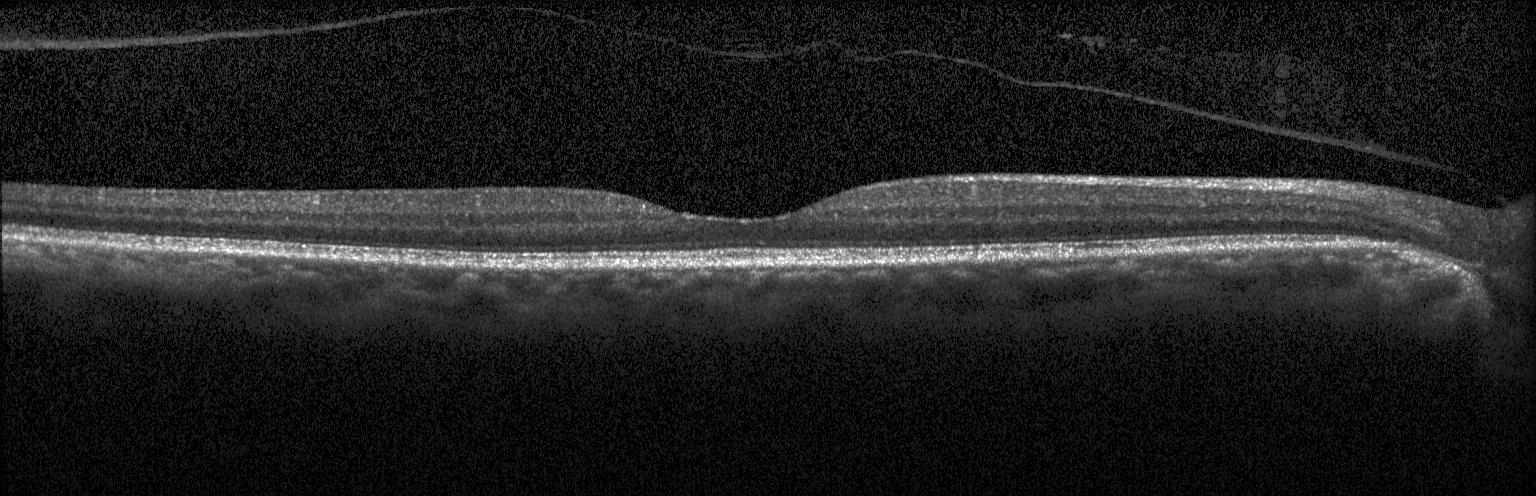

Finding: no evidence of choroidal neovascularization, diabetic macular edema, or drusen.